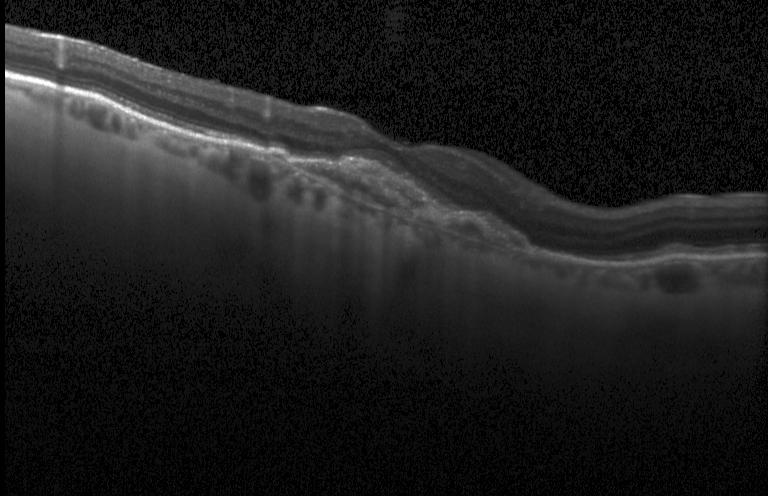 Dx: choroidal neovascularization (CNV).